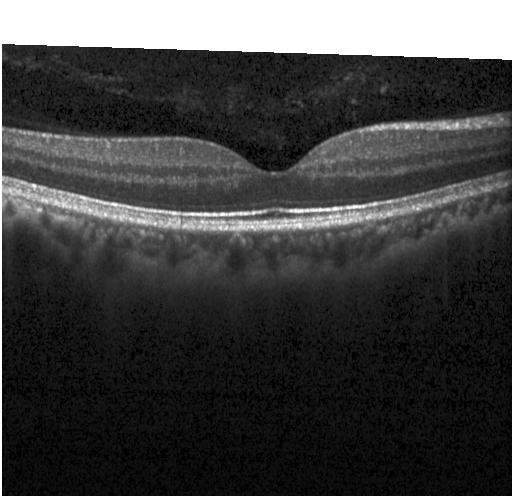

SD-OCT, acquired on a Heidelberg Spectralis, OCT line scan
The scan shows no choroidal neovascularization, no diabetic macular edema, and no drusen.